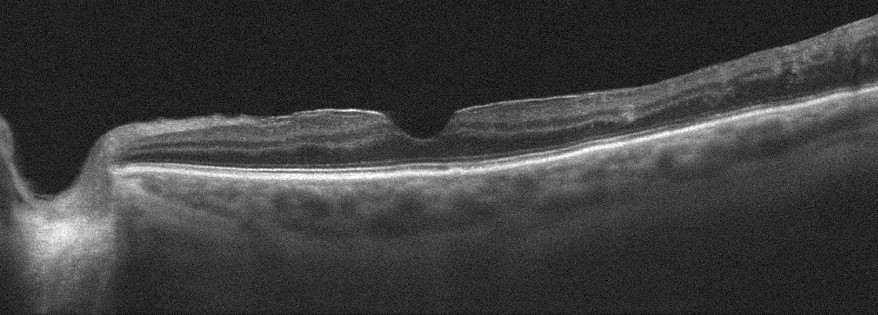
This B-scan demonstrates epiretinal membrane.